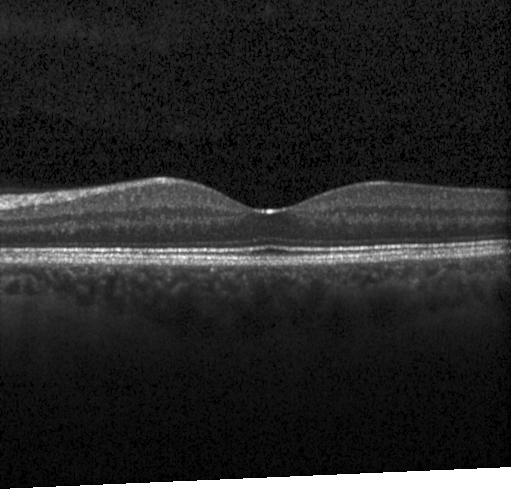
Macular OCT demonstrating no evidence of CNV, DME, or drusen.